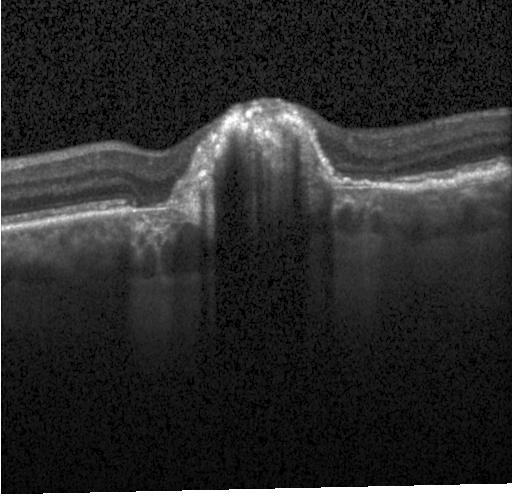
Optical coherence tomography scan, acquired on a Heidelberg Spectralis, spectral-domain OCT.
Impression: choroidal neovascularization (CNV).